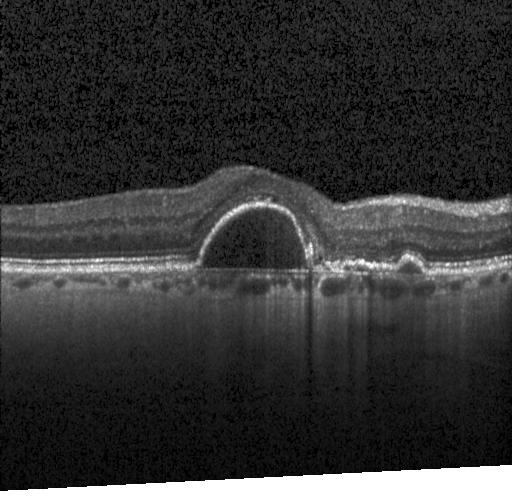 The scan shows a choroidal neovascular membrane.